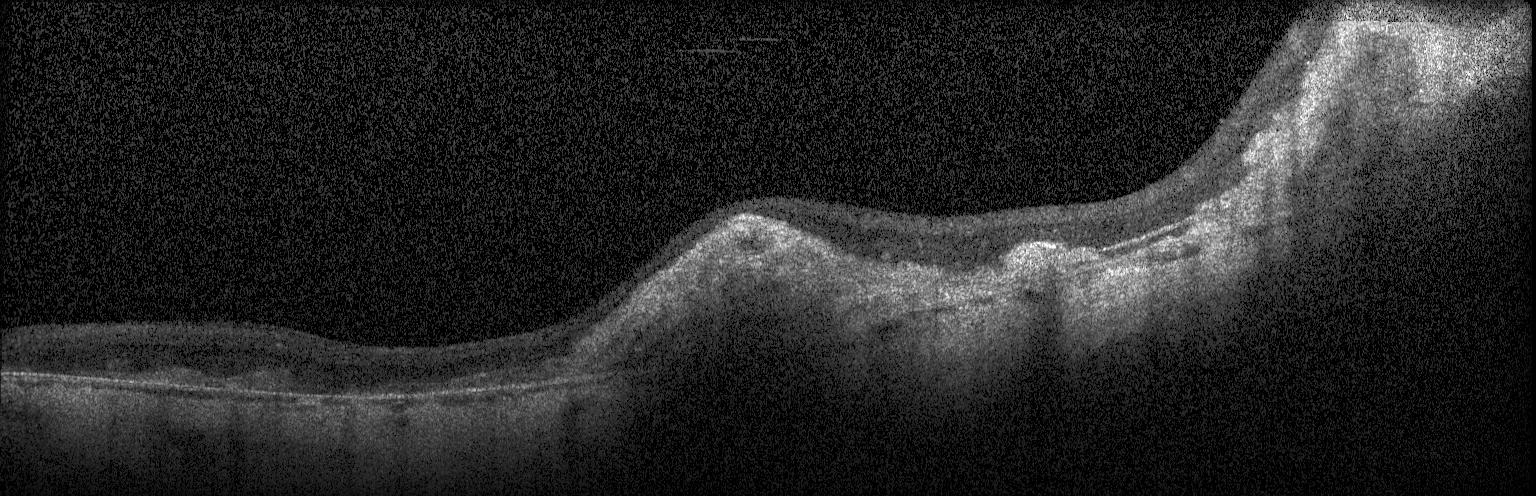

Spectral-domain optical coherence tomography. Retinal OCT B-scan.
Finding: choroidal neovascularization (CNV).